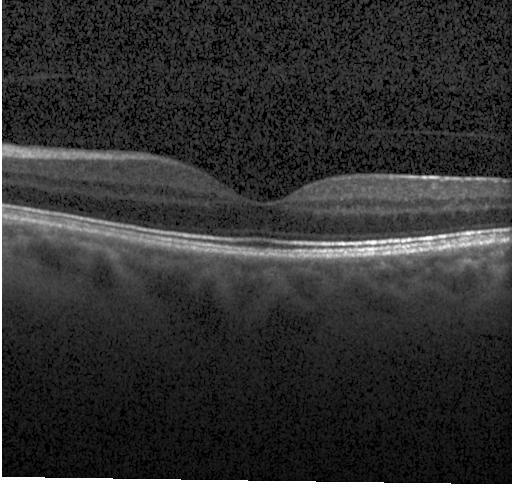
Optical coherence tomography scan, through the macula, acquired on a Heidelberg Spectralis, SD-OCT — Finding: no choroidal neovascularization, no diabetic macular edema, and no drusen.